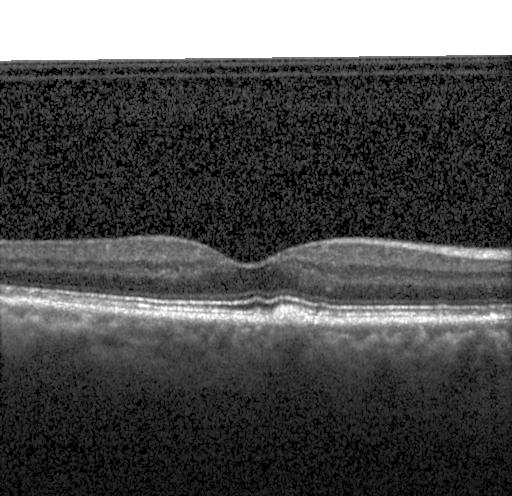 Spectral-domain optical coherence tomography. Retinal OCT cross-section. Heidelberg Spectralis. Dx: drusen.